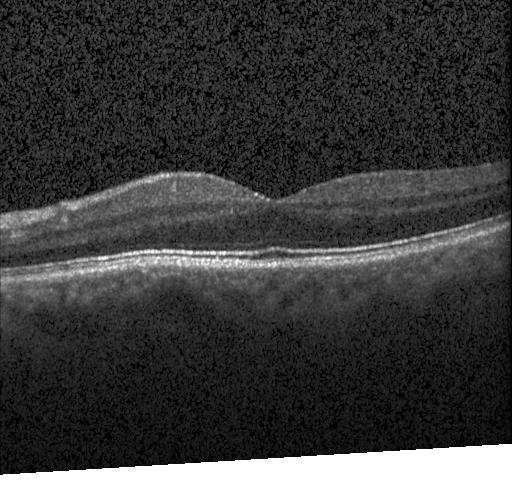 Optical coherence tomography scan · macular scan.
Finding: neither choroidal neovascularization, diabetic macular edema, nor drusen.